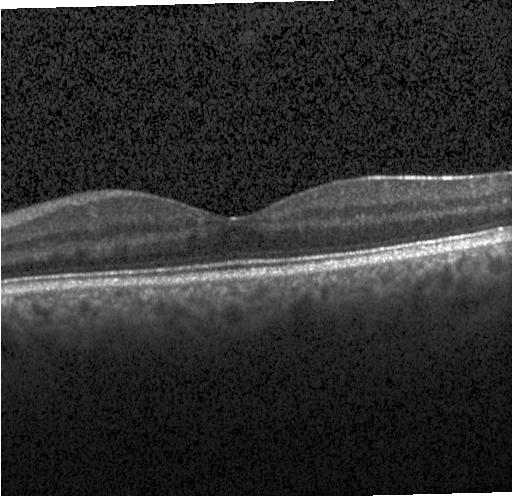
Finding: no choroidal neovascularization, diabetic macular edema, or drusen.